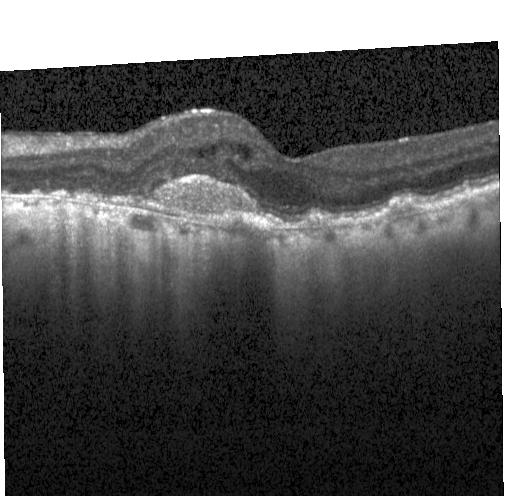
Impression: a choroidal neovascular membrane.